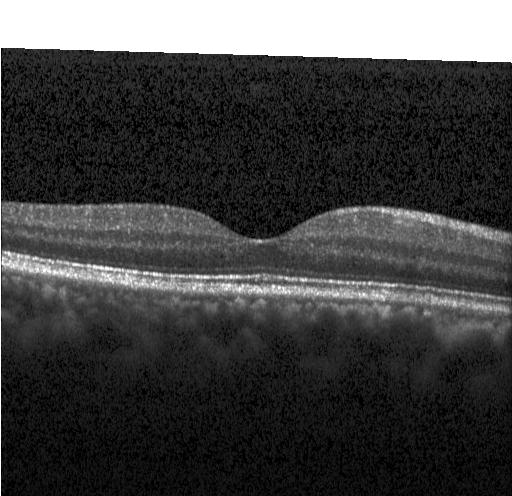 Heidelberg Spectralis OCT system, OCT line scan
Diagnosis: no CNV, DME, or drusen.